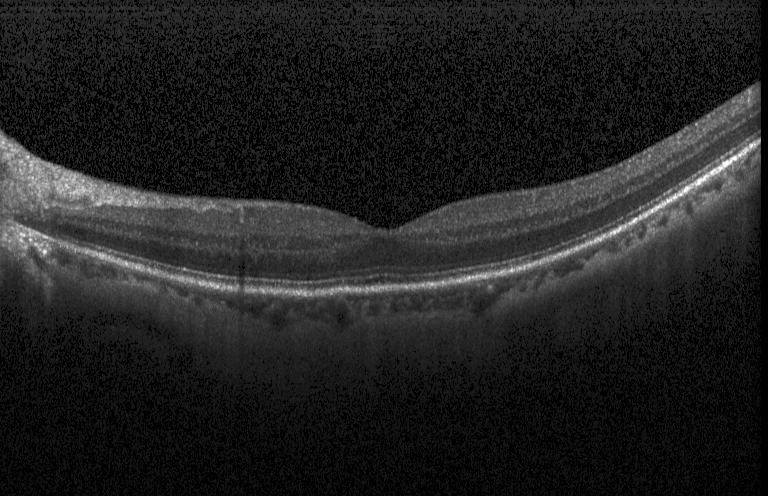
Acquired on a Heidelberg Spectralis · SD-OCT · optical coherence tomography scan.
The scan shows no evidence of choroidal neovascularization, diabetic macular edema, or drusen.